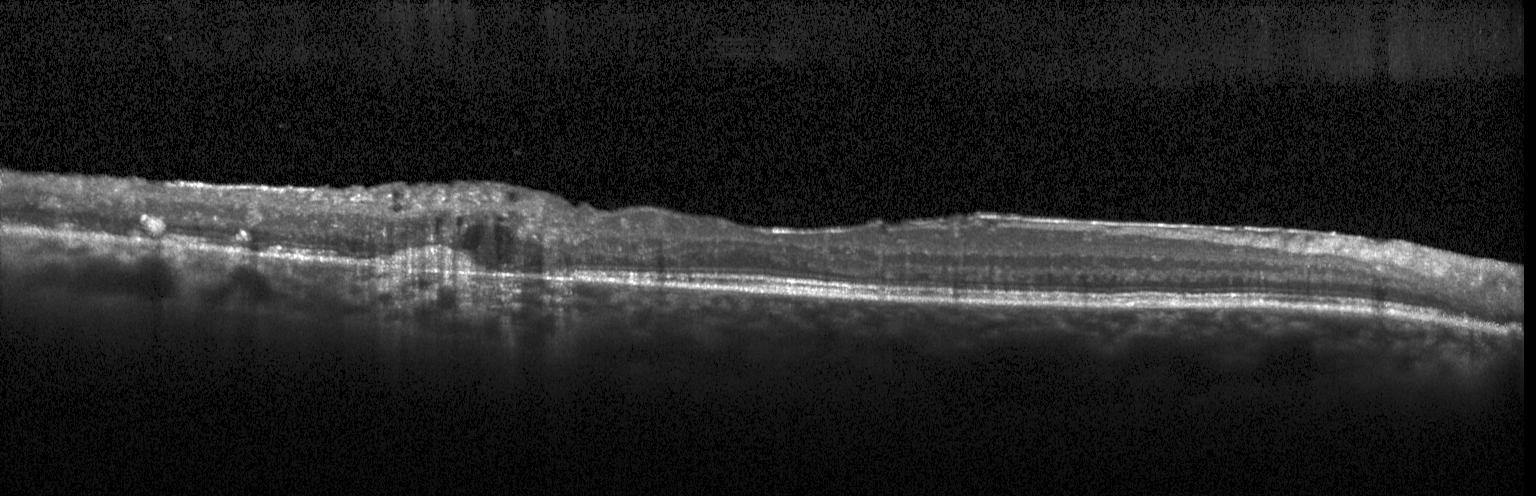 Diagnosis: a choroidal neovascular membrane.